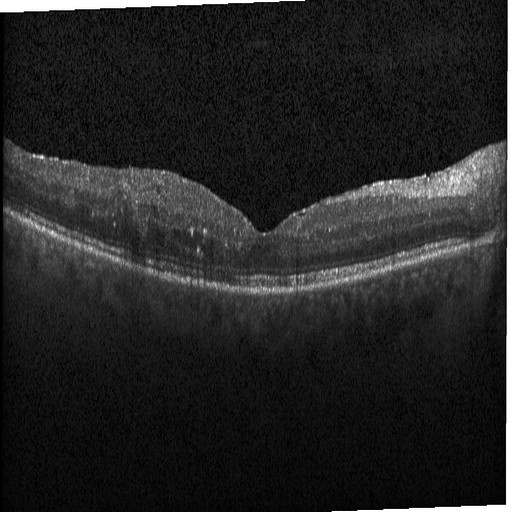

Retinal OCT cross-section; fovea-centered; spectral-domain optical coherence tomography; Heidelberg Spectralis.
Diagnosis: diabetic macular edema.